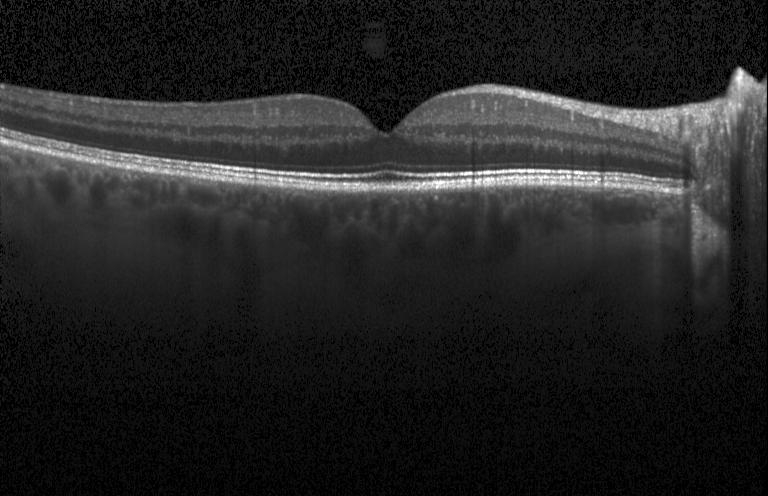 Spectral-domain OCT. Retinal OCT B-scan. Acquired on a Heidelberg Spectralis. Fovea-centered — Assessment: no choroidal neovascularization, no diabetic macular edema, and no drusen.